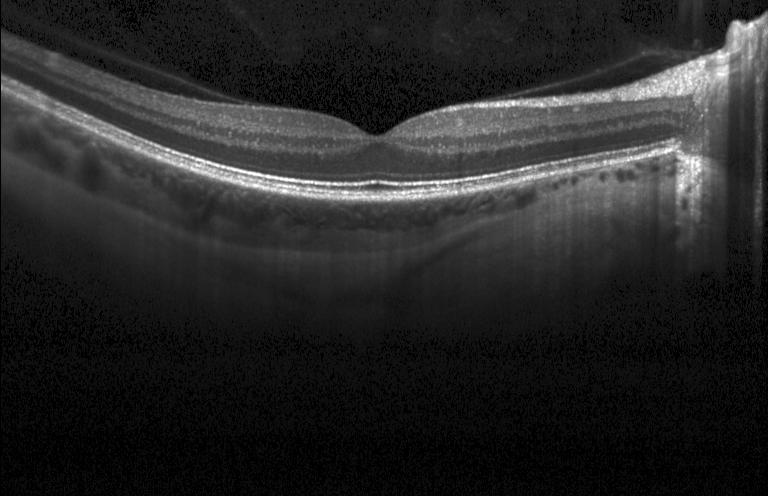 Retinal OCT cross-section; macular scan — Impression: no CNV, DME, or drusen.